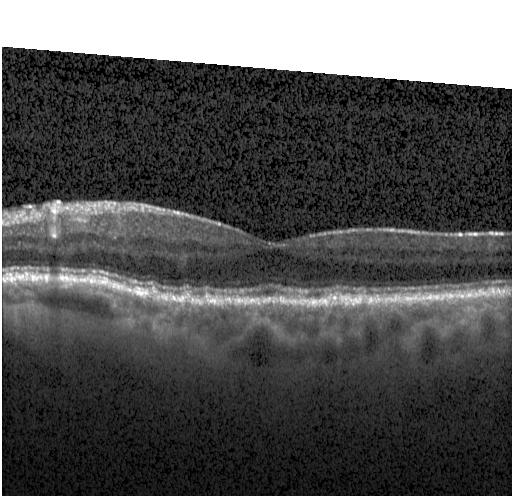
Finding: drusen.